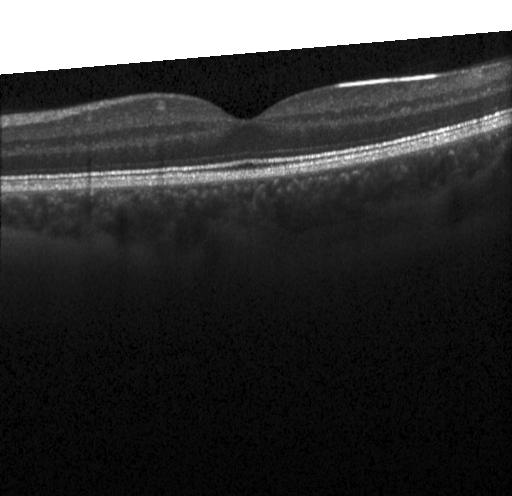 Macular OCT: no CNV, DME, or drusen.